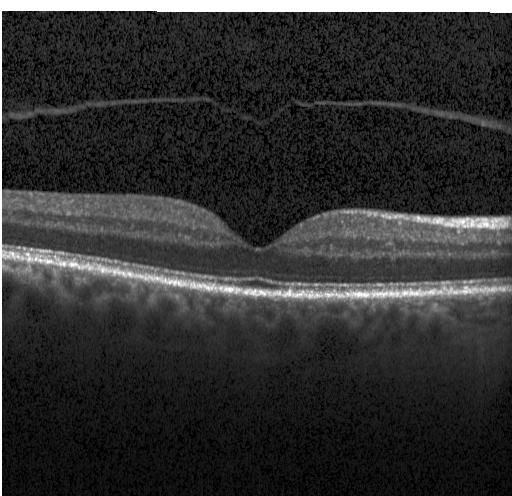

Dx: neither CNV, DME, nor drusen.